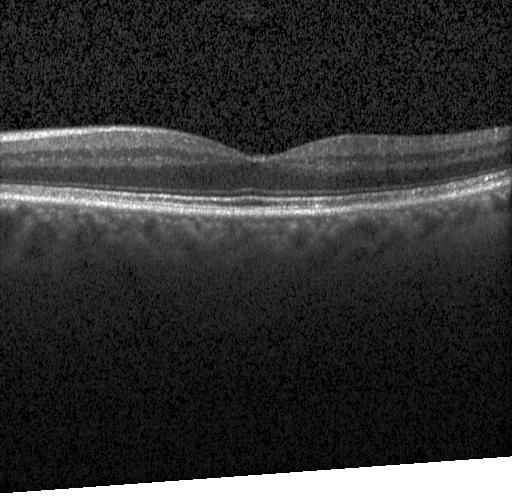
Retinal OCT B-scan, SD-OCT, acquired on a Heidelberg Spectralis
Impression: no evidence of choroidal neovascularization, diabetic macular edema, or drusen.